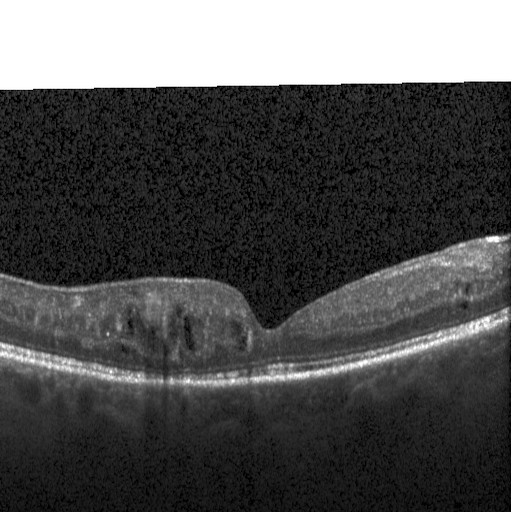
Retinal OCT B-scan, Heidelberg Spectralis OCT system
Impression: DME.